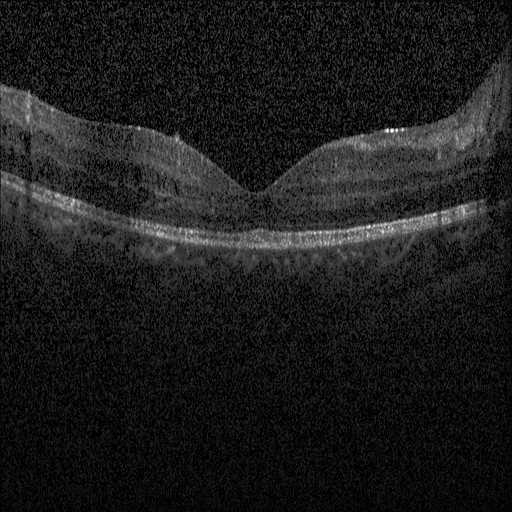

Retinal OCT B-scan, instrument: Heidelberg Spectralis, spectral-domain optical coherence tomography. Diagnosis: diabetic macular edema (DME).